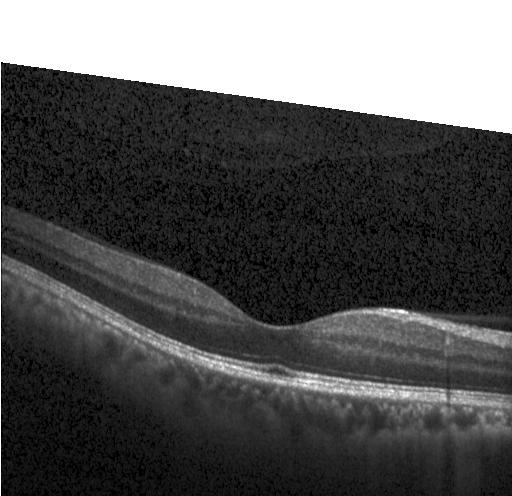 This B-scan demonstrates no evidence of choroidal neovascularization, diabetic macular edema, or drusen.